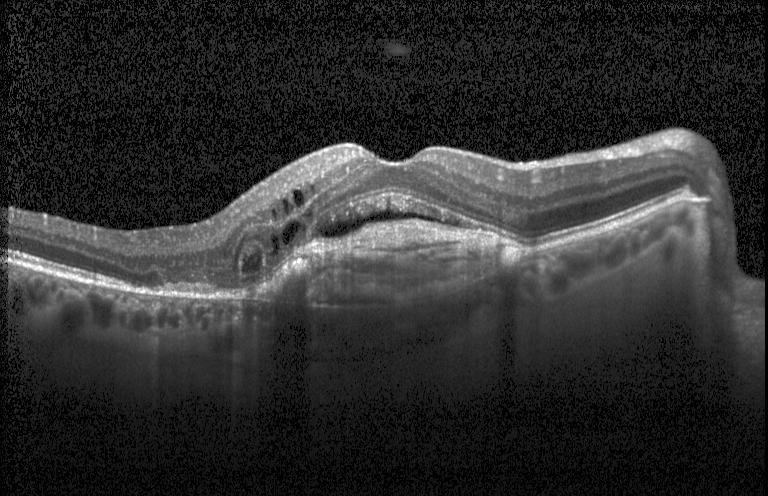

Macular scan · OCT B-scan.
Finding: choroidal neovascularization.